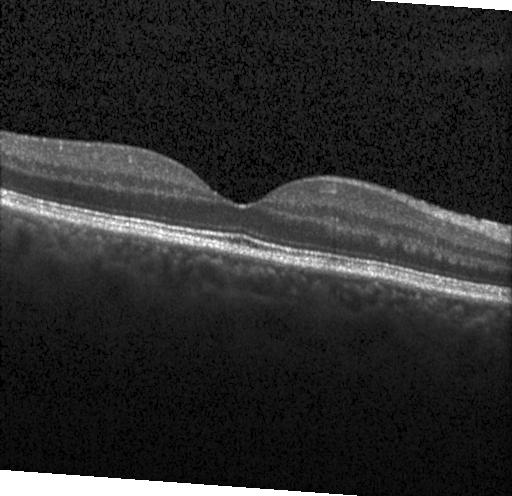
Impression: no CNV, DME, or drusen.